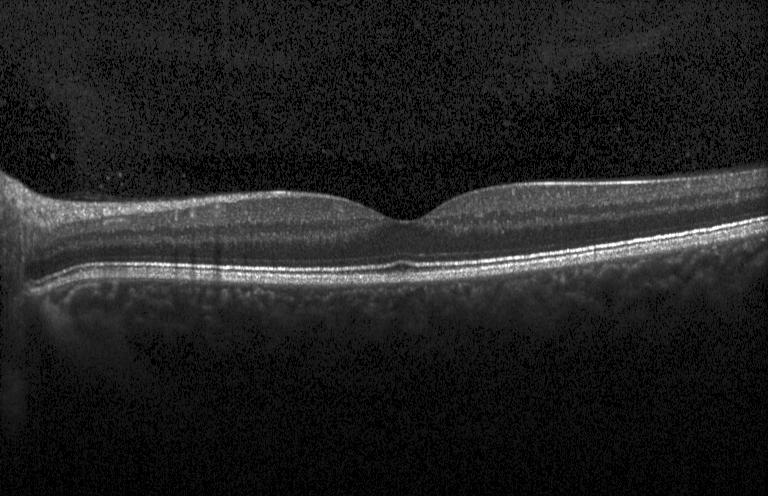 Spectral-domain OCT B-scan: neither choroidal neovascularization, diabetic macular edema, nor drusen.